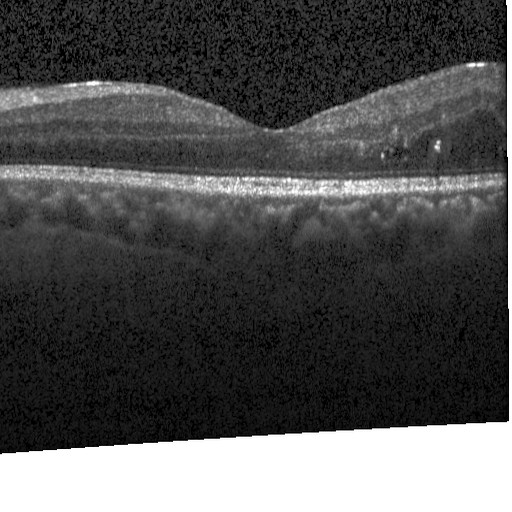 Retinal OCT cross-section showing diabetic macular edema.